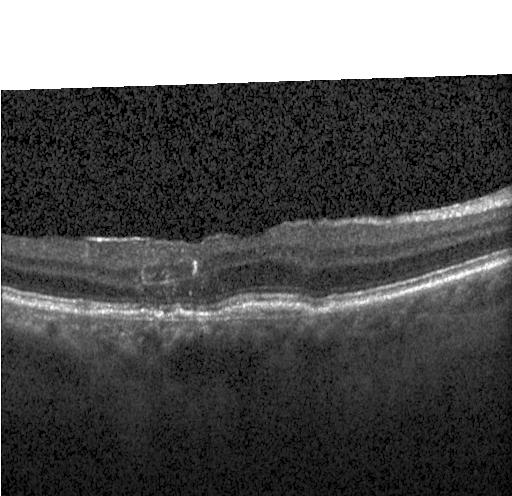
Macular scan · Heidelberg Spectralis · spectral-domain OCT · optical coherence tomography scan — Assessment: a choroidal neovascular membrane.